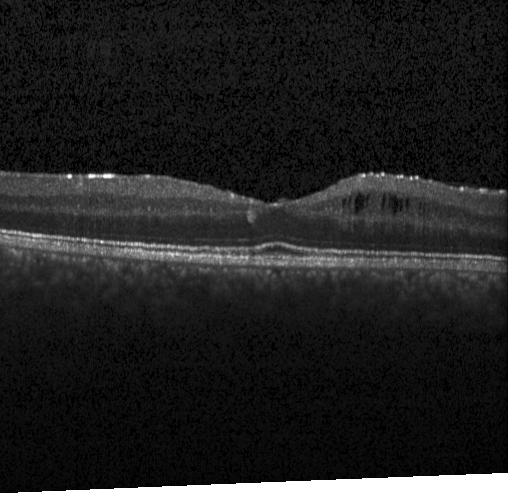 DME.